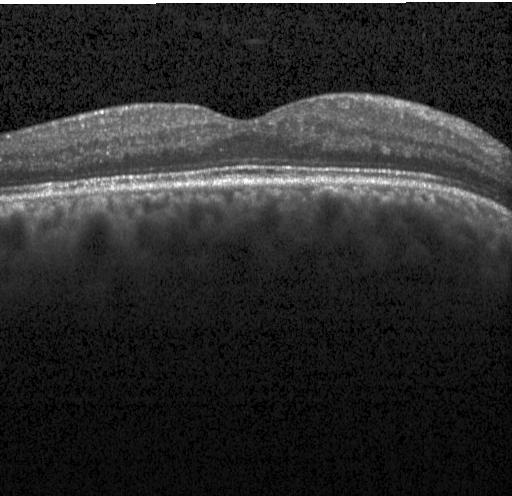
Impression: no choroidal neovascularization, diabetic macular edema, or drusen.